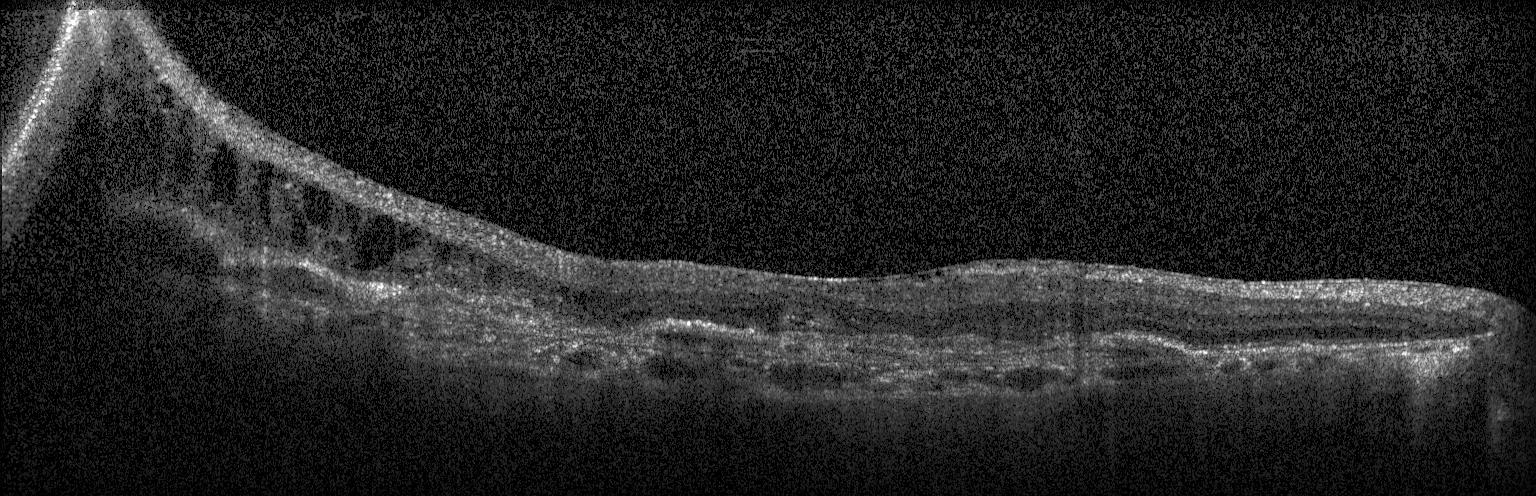

Optical coherence tomography B-scan. This B-scan demonstrates a choroidal neovascular membrane.